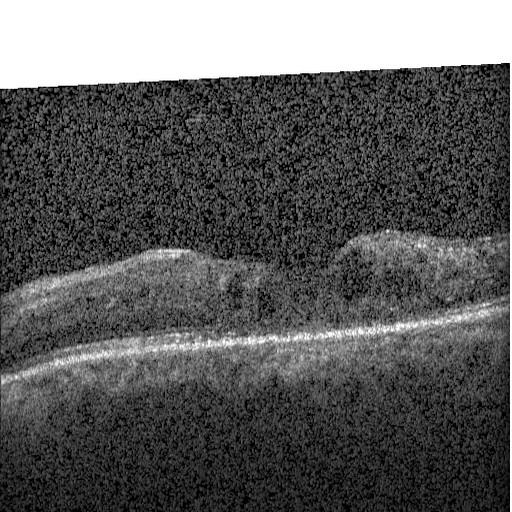

Retinal OCT cross-section.
The scan shows diabetic macular edema.